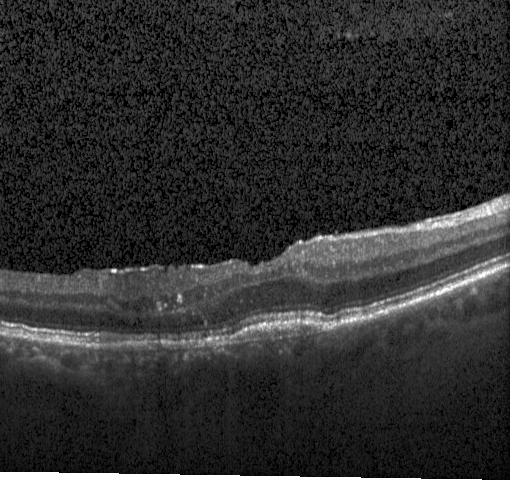
The scan shows a choroidal neovascular membrane.